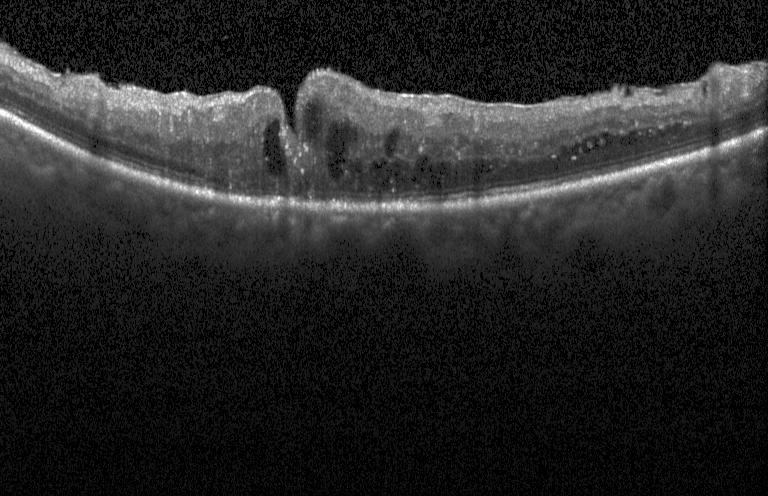

Retinal OCT cross-section
Dx: diabetic macular edema.